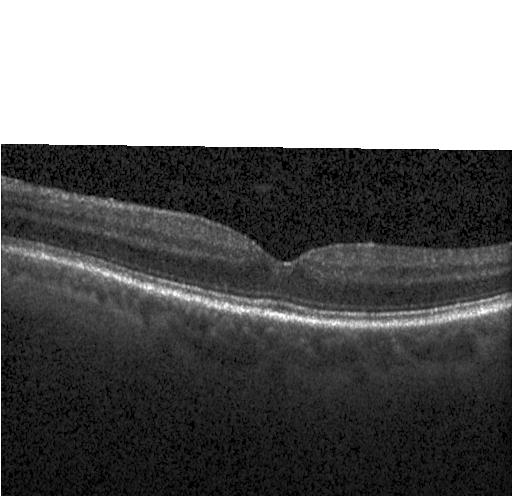
Retinal OCT cross-section showing neither CNV, DME, nor drusen.